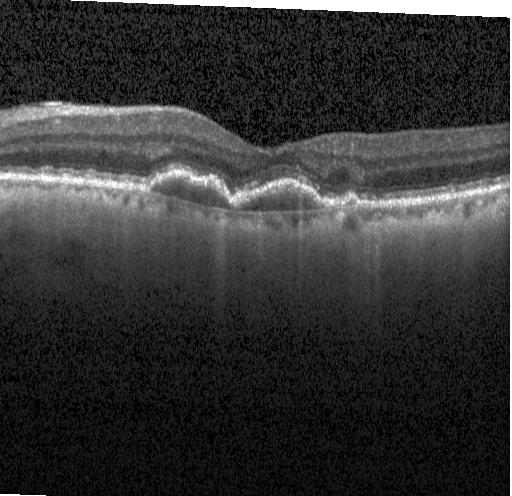 Retinal OCT B-scan, instrument: Heidelberg Spectralis, macular scan, spectral-domain OCT.
Finding: choroidal neovascularization.